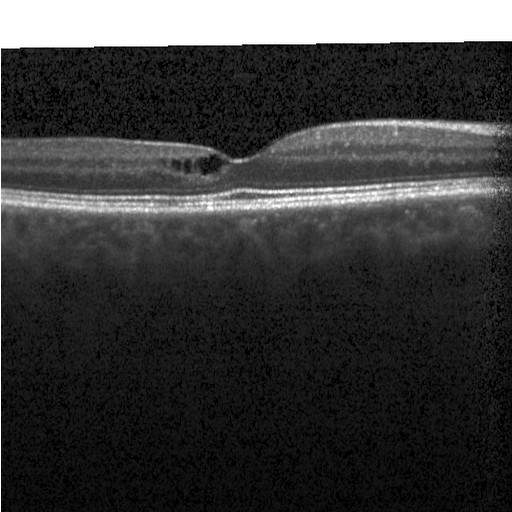 Spectral-domain OCT · through the macula · OCT line scan · Heidelberg Spectralis OCT system. Finding: DME.